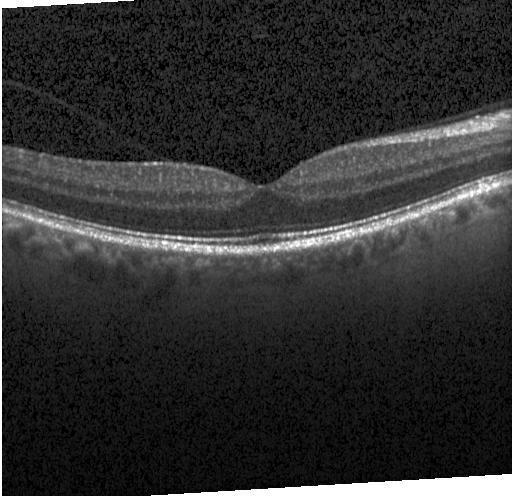

Macular OCT: no choroidal neovascularization, diabetic macular edema, or drusen.